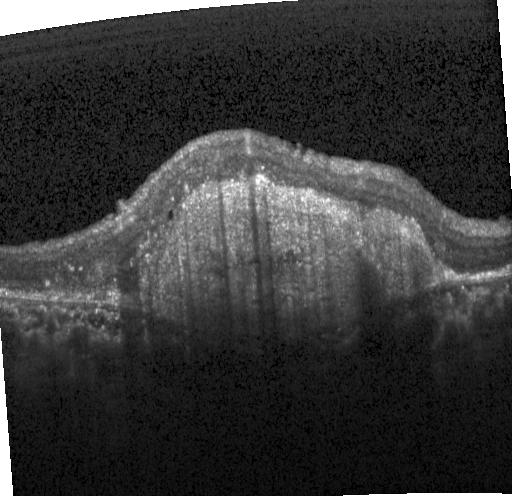 Fovea-centered. Heidelberg Spectralis OCT system. Optical coherence tomography scan
OCT finding: CNV.